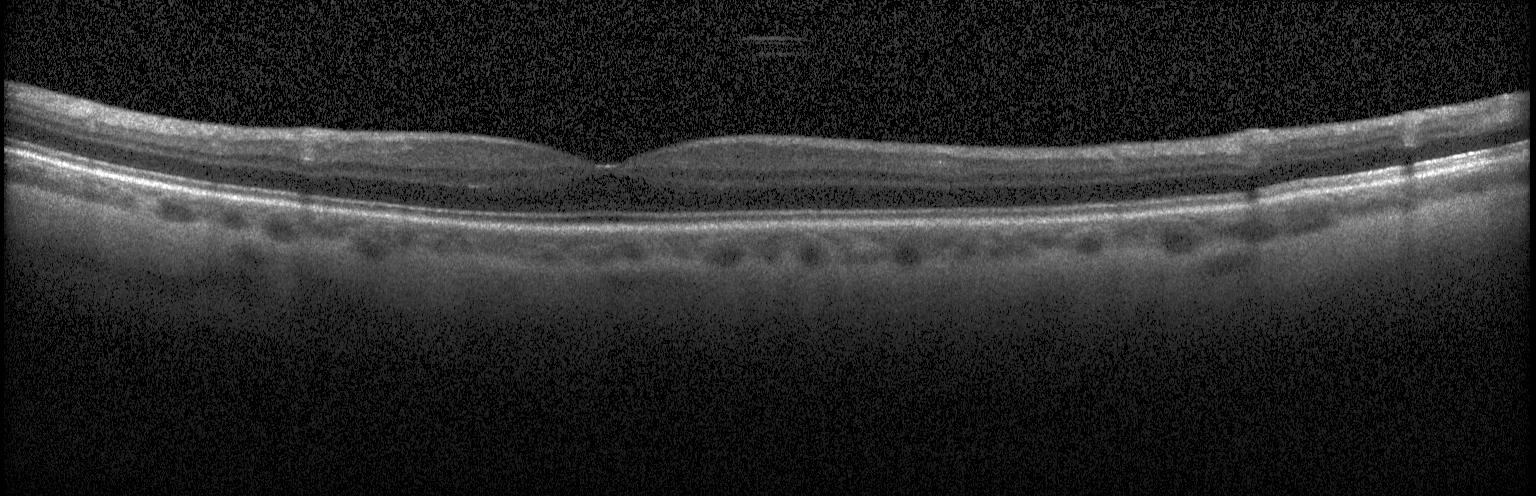

Horizontal scan through the fovea; retinal OCT B-scan; Heidelberg Spectralis OCT system; spectral-domain optical coherence tomography
Assessment: no CNV, DME, or drusen.